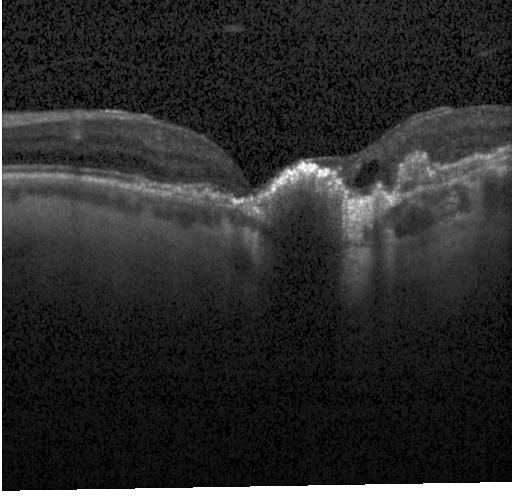
Macular OCT: choroidal neovascularization.